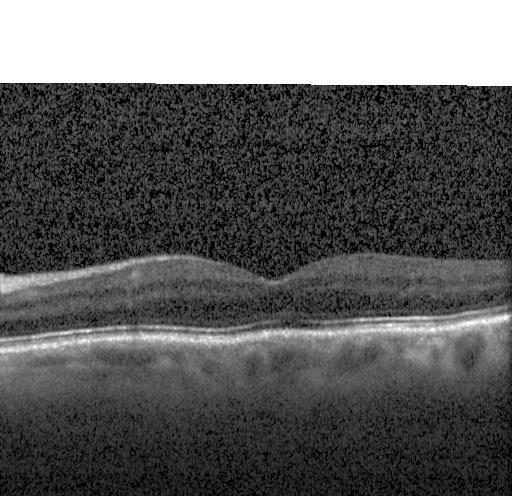
Optical coherence tomography B-scan. The scan shows no CNV, no DME, and no drusen.